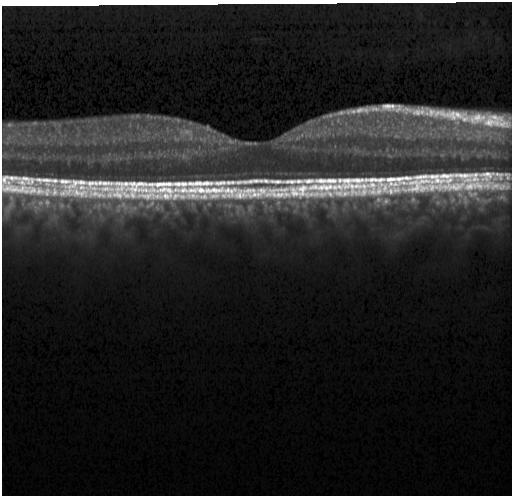 Finding: no evidence of CNV, DME, or drusen.